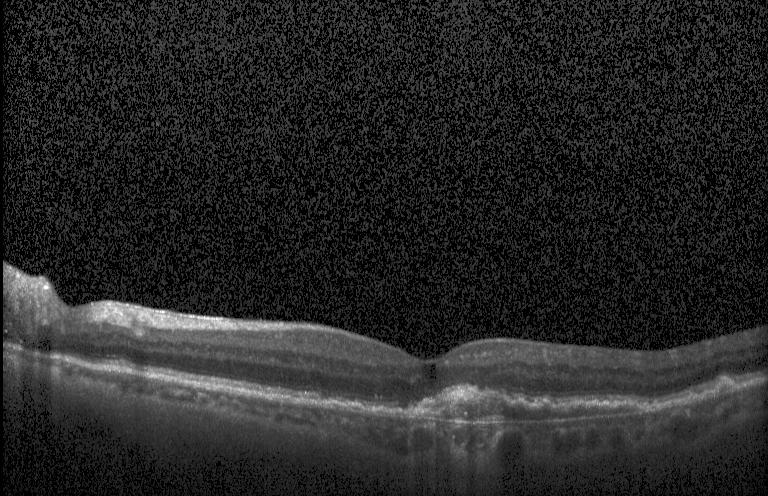
OCT scan showing choroidal neovascularization (CNV).